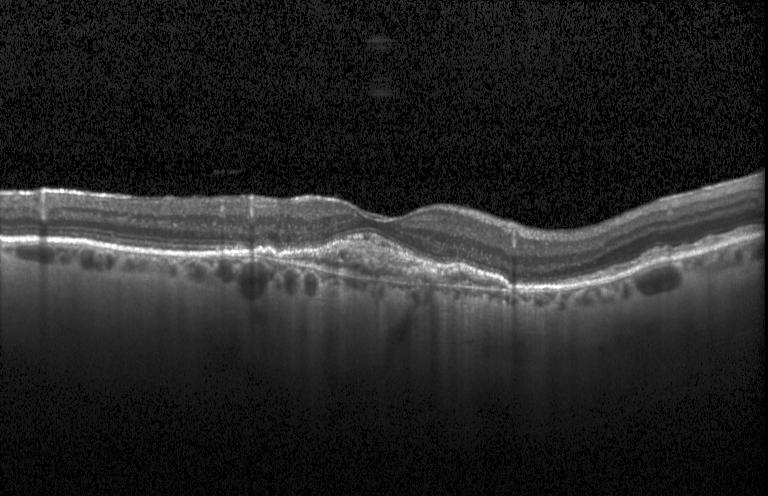
Acquired on a Heidelberg Spectralis. Horizontal scan through the fovea. Retinal OCT cross-section. Macular OCT: a choroidal neovascular membrane.